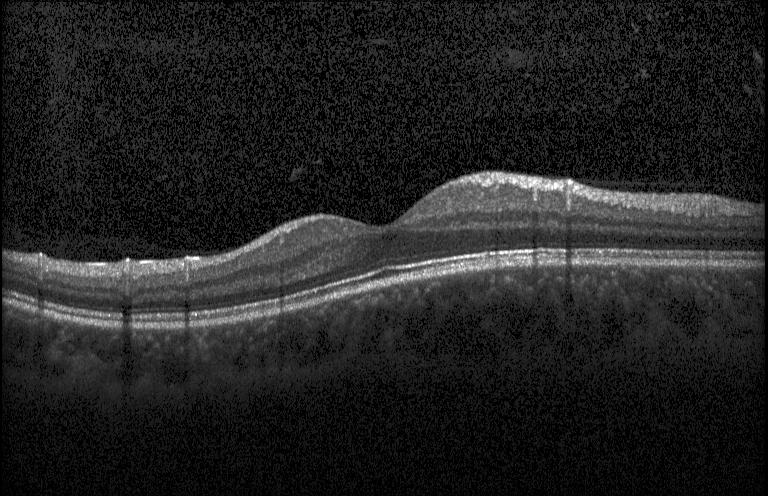 Retinal OCT cross-section showing neither choroidal neovascularization, diabetic macular edema, nor drusen.